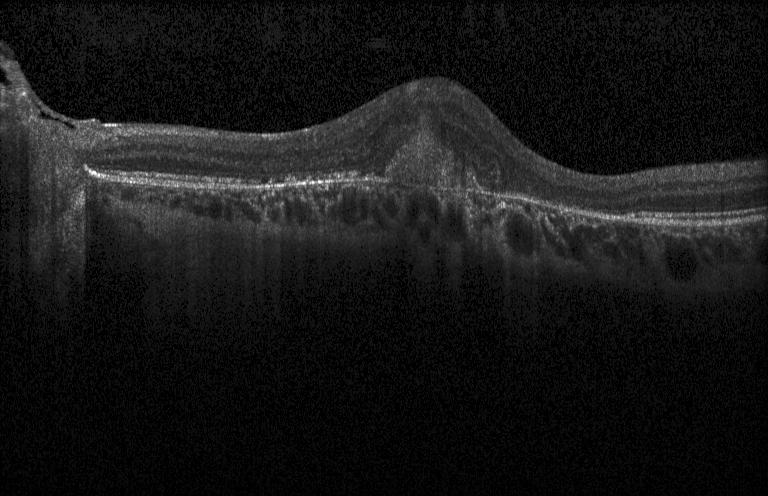

SD-OCT · OCT line scan — The scan shows a choroidal neovascular membrane.